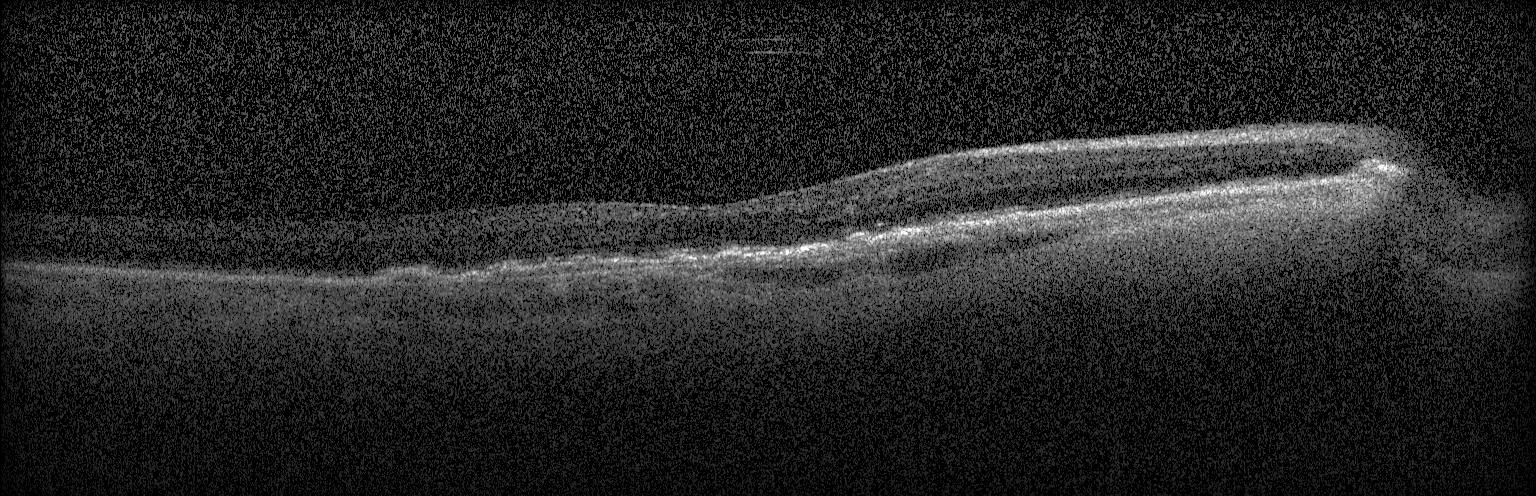

Optical coherence tomography scan.
Dx: a choroidal neovascular membrane.